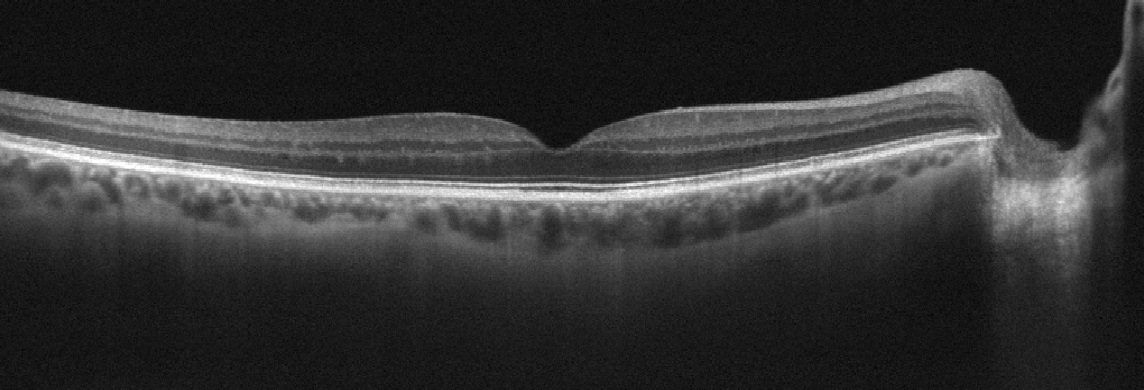 The scan shows no evidence of AMD, DME, ERM, RAO, RVO, or VID.